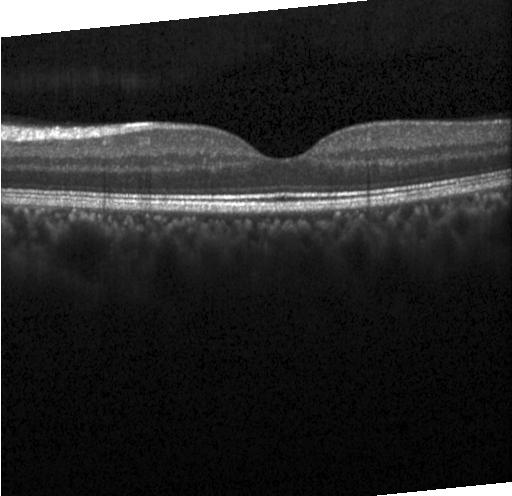
OCT B-scan
Macular OCT: no choroidal neovascularization, no diabetic macular edema, and no drusen.